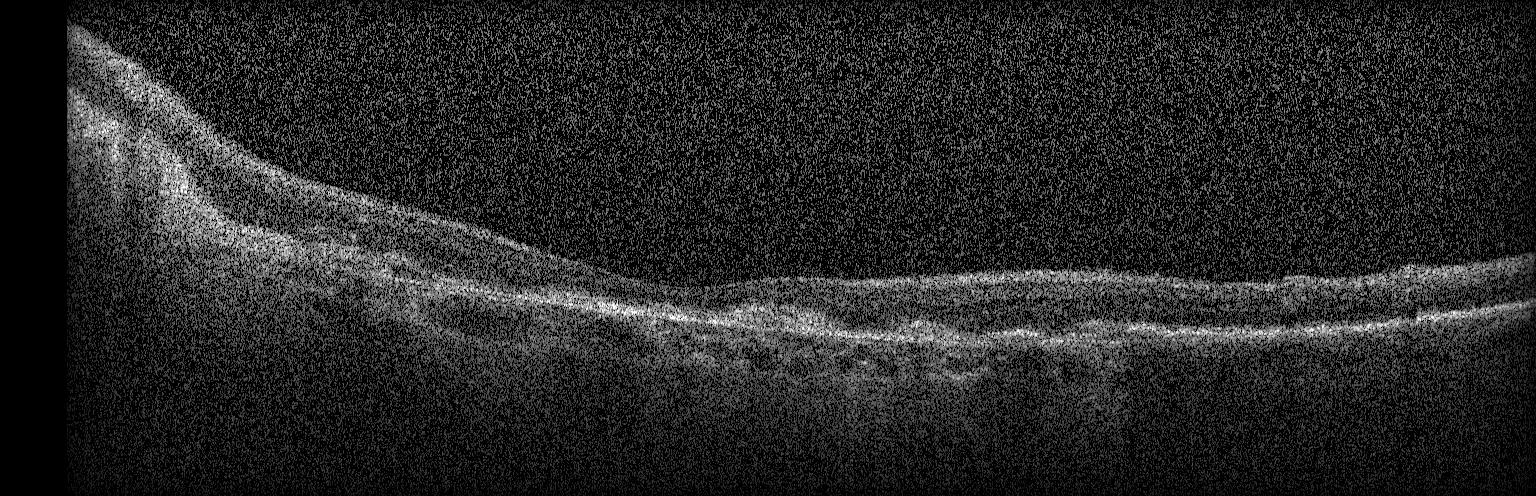 Macular OCT: choroidal neovascularization.